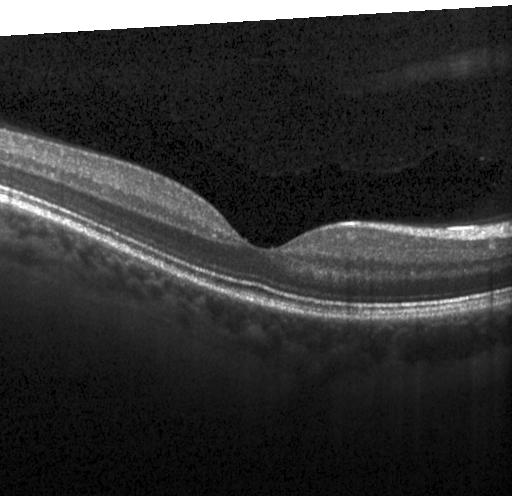
OCT line scan
OCT finding: no choroidal neovascularization, no diabetic macular edema, and no drusen.